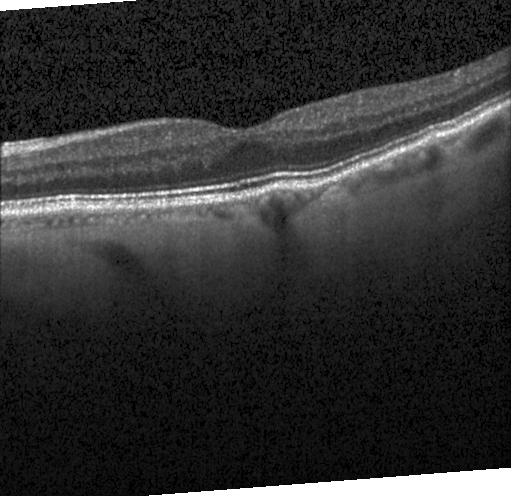
Retinal OCT cross-section.
OCT finding: no evidence of CNV, DME, or drusen.